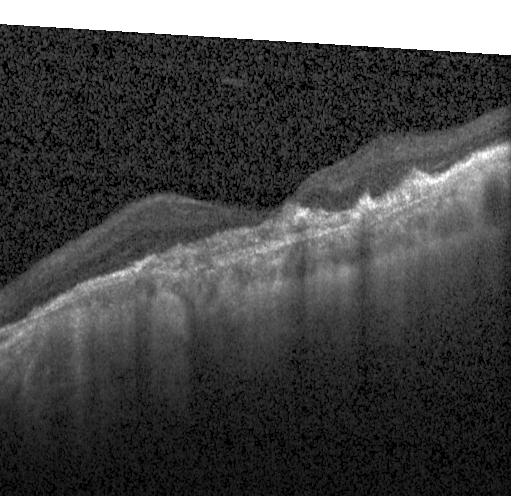

Heidelberg Spectralis OCT system, spectral-domain OCT, OCT B-scan
Impression: CNV.